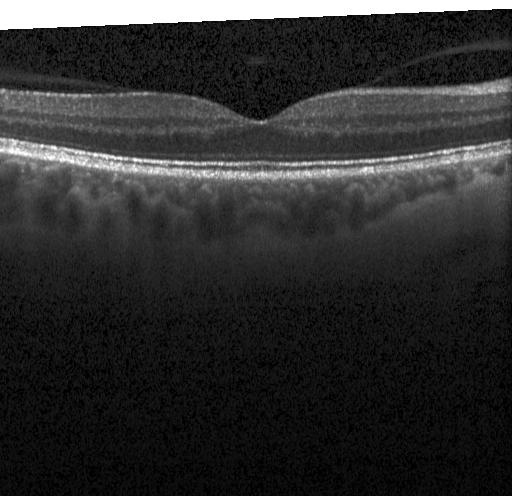
Optical coherence tomography scan. Diagnosis: no choroidal neovascularization, no diabetic macular edema, and no drusen.